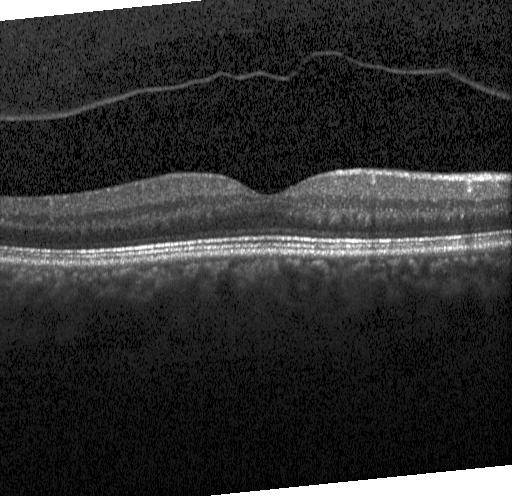
Spectral-domain optical coherence tomography. Optical coherence tomography scan. Heidelberg Spectralis OCT system — Finding: no choroidal neovascularization, diabetic macular edema, or drusen.